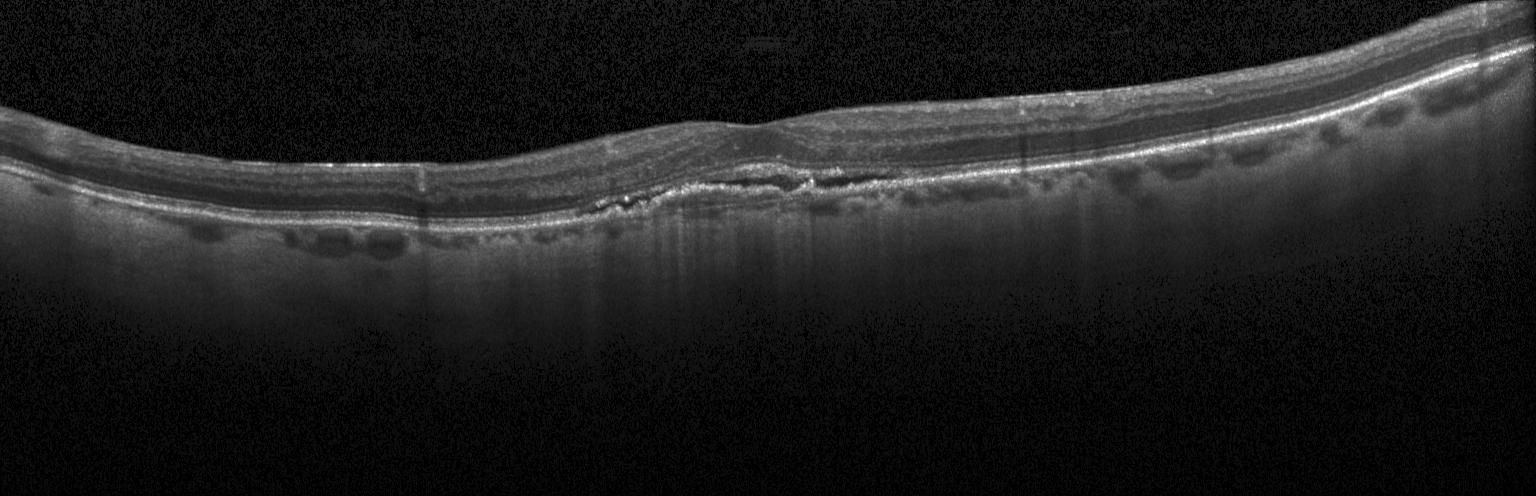

Macular OCT: a choroidal neovascular membrane.